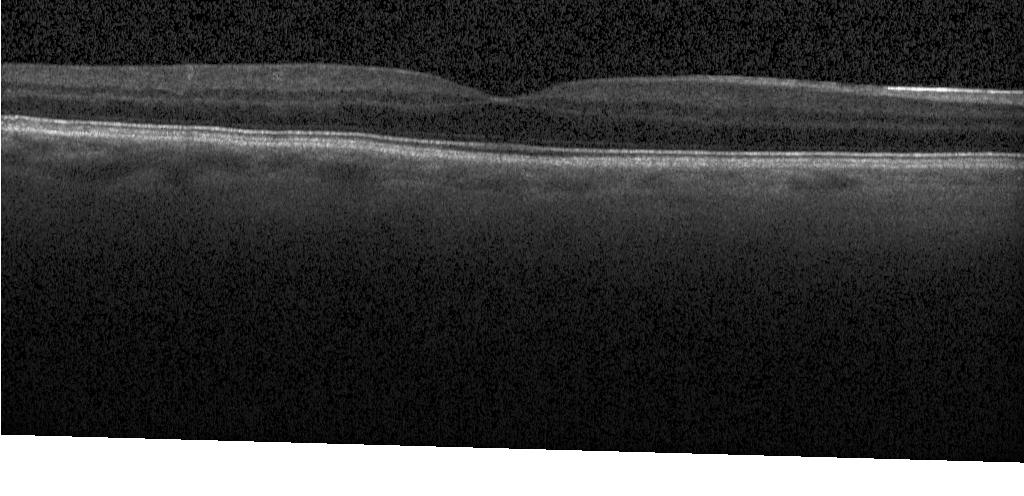
Spectral-domain OCT, retinal OCT cross-section
OCT finding: neither choroidal neovascularization, diabetic macular edema, nor drusen.